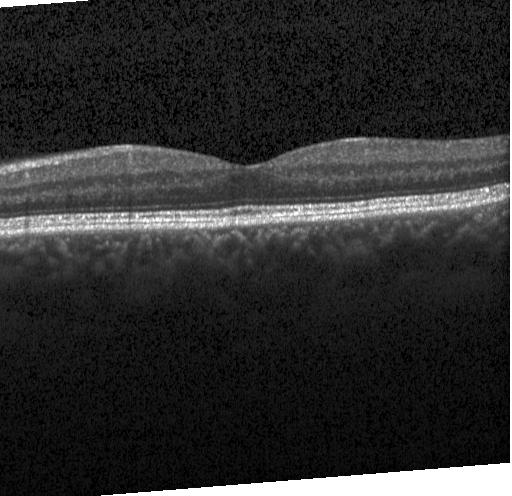 Macular scan · SD-OCT · Heidelberg Spectralis OCT system · OCT B-scan. Finding: neither choroidal neovascularization, diabetic macular edema, nor drusen.